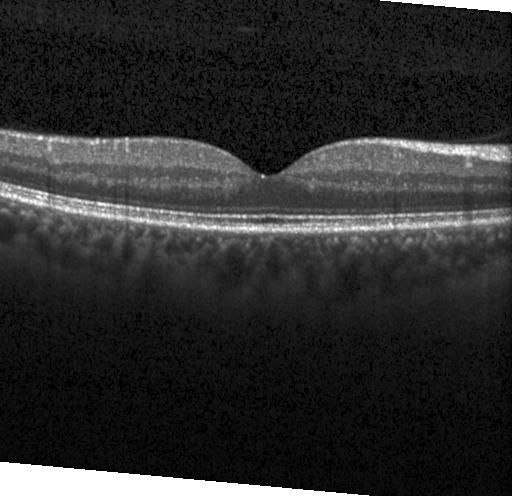 Spectral-domain OCT B-scan: no evidence of choroidal neovascularization, diabetic macular edema, or drusen.